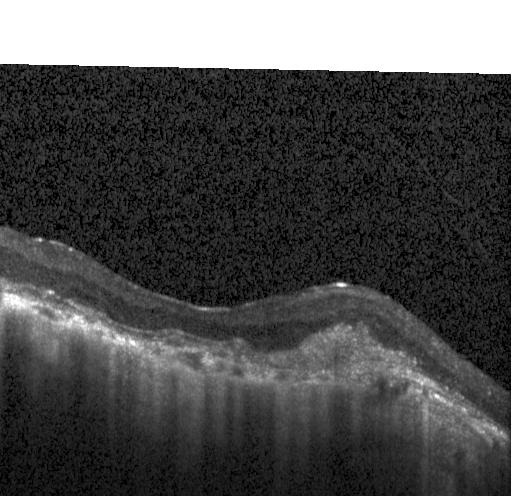 Finding: a choroidal neovascular membrane.